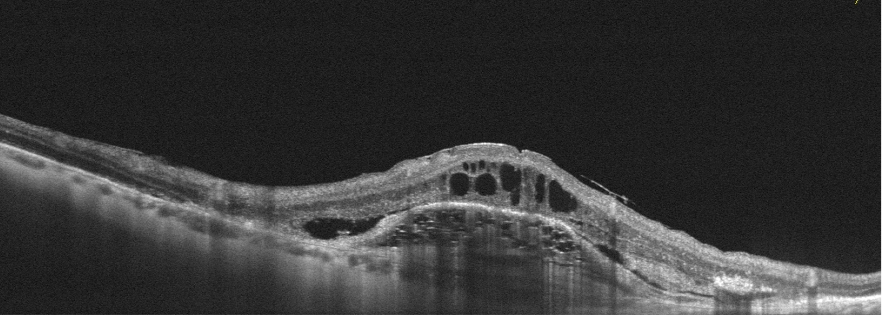

Optovue Avanti RTVue XR · retinal OCT cross-section
OCT finding: age-related macular degeneration.